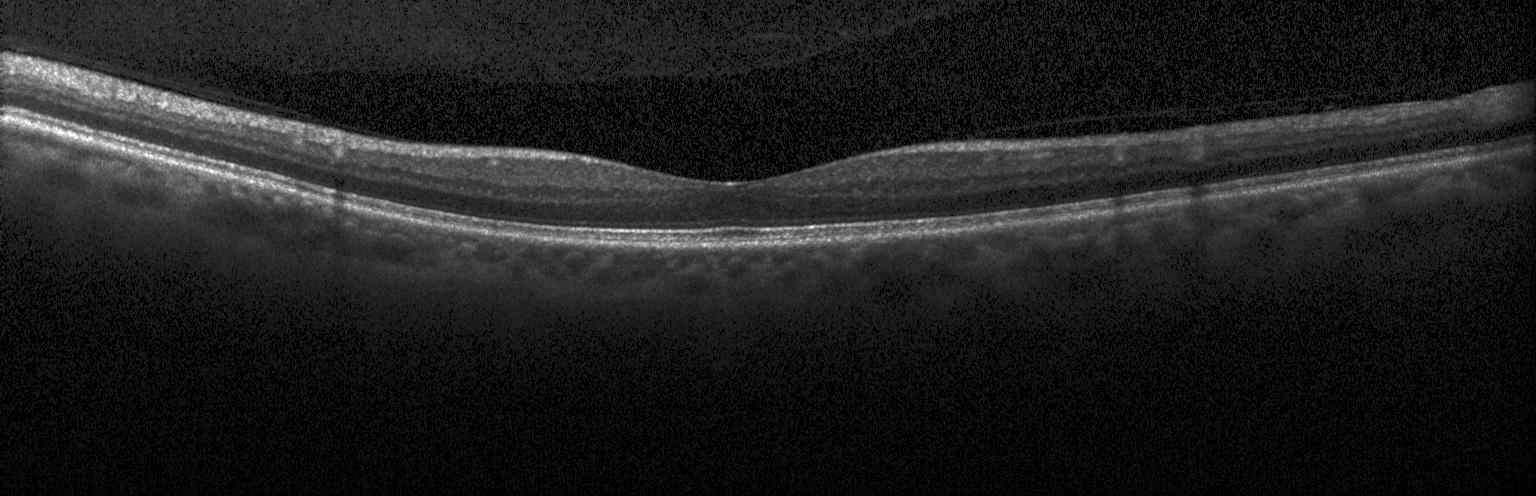

Retinal OCT B-scan; instrument: Heidelberg Spectralis.
Dx: no evidence of choroidal neovascularization, diabetic macular edema, or drusen.